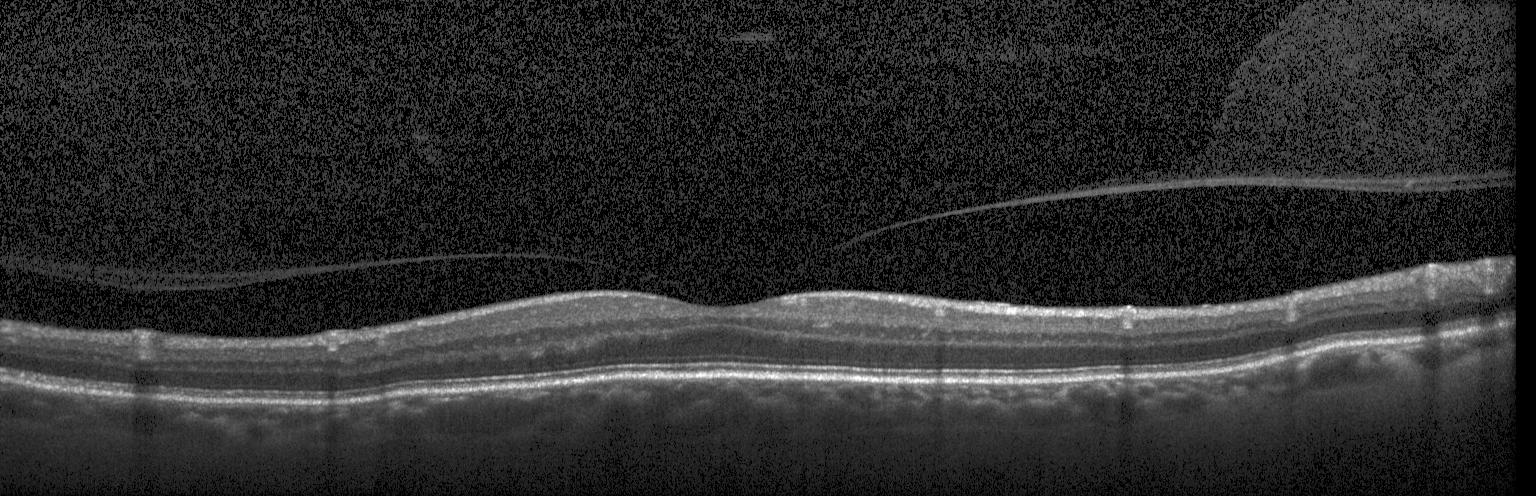 Macular OCT: no choroidal neovascularization, diabetic macular edema, or drusen.